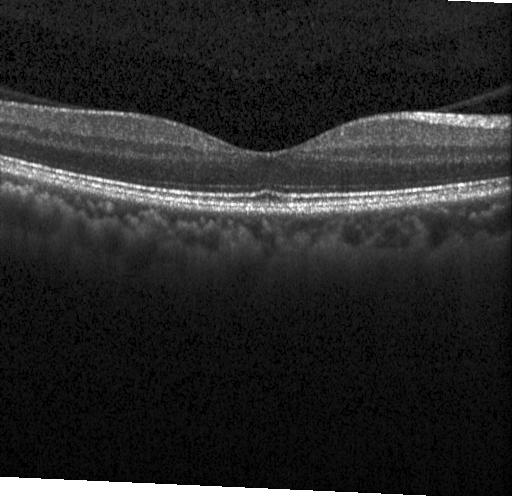 Macular scan, SD-OCT, Heidelberg Spectralis, optical coherence tomography scan
Dx: no choroidal neovascularization, diabetic macular edema, or drusen.